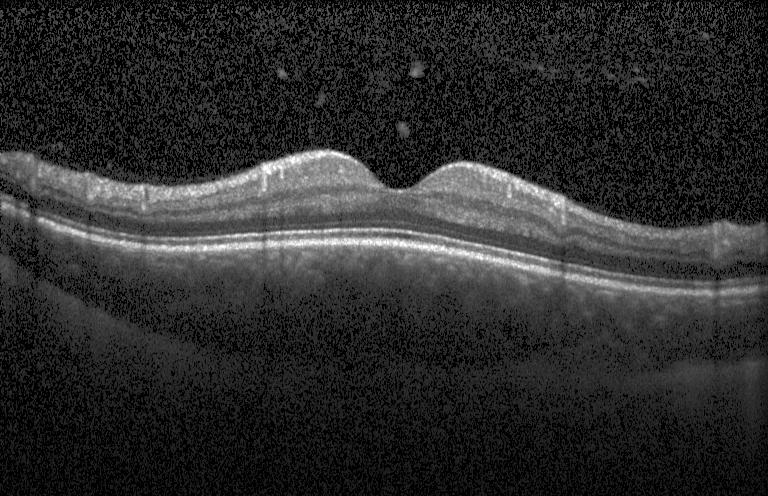

Optical coherence tomography B-scan.
This B-scan demonstrates no evidence of CNV, DME, or drusen.